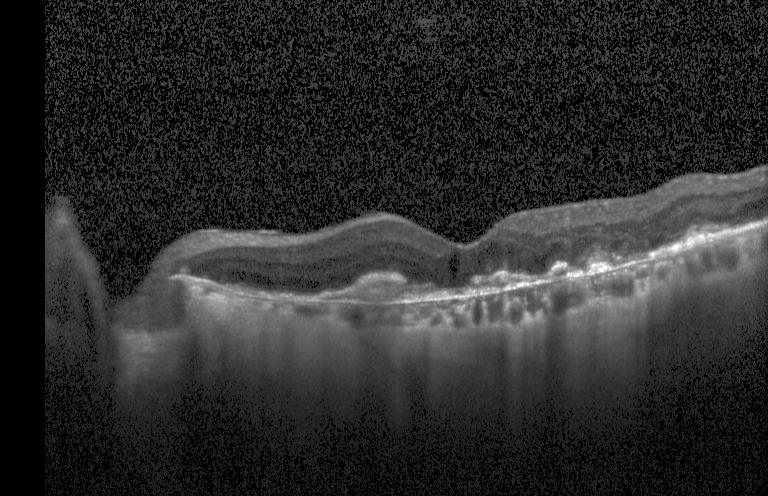

Dx: a choroidal neovascular membrane.